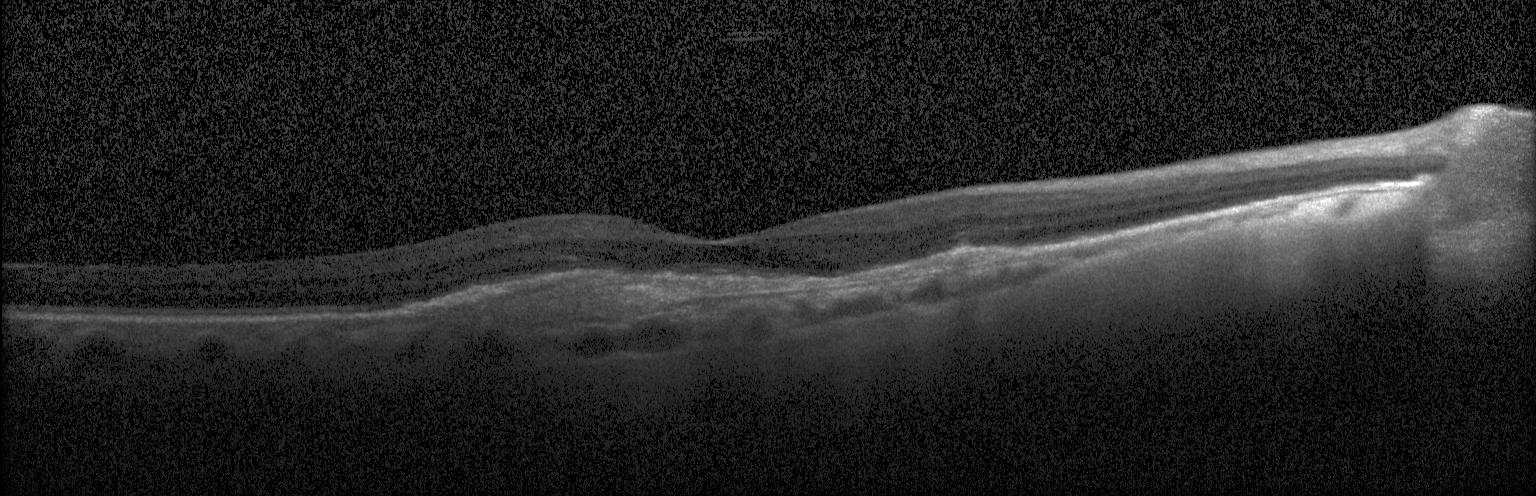 Horizontal scan through the fovea; SD-OCT; instrument: Heidelberg Spectralis; OCT B-scan — OCT finding: choroidal neovascularization.